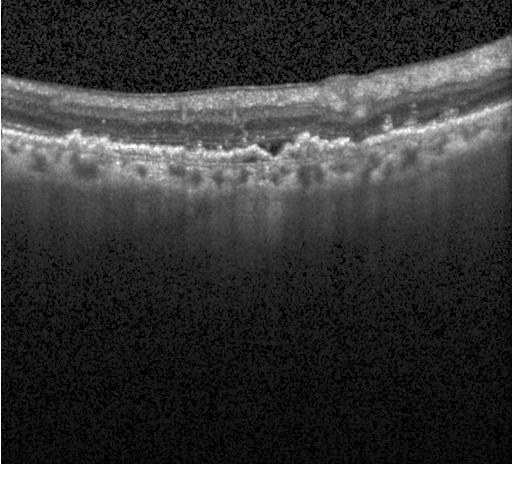
OCT B-scan; SD-OCT; Heidelberg Spectralis OCT system; through the macula.
Assessment: choroidal neovascularization (CNV).